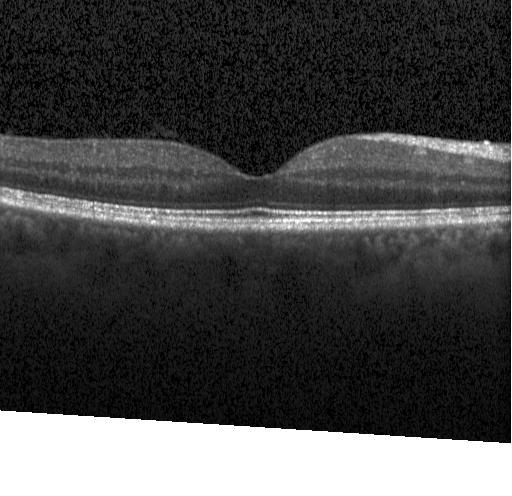

Optical coherence tomography scan. Assessment: no choroidal neovascularization, diabetic macular edema, or drusen.